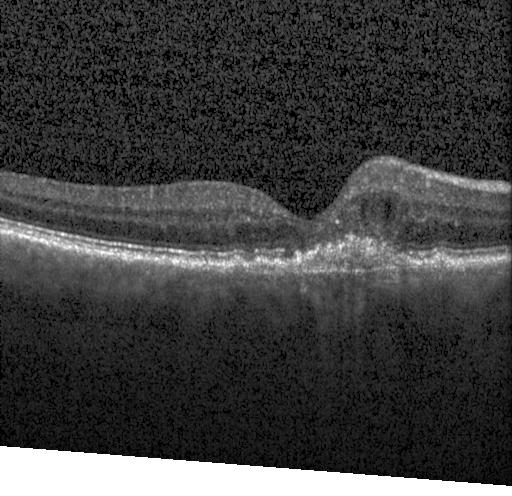
OCT B-scan; SD-OCT. Assessment: choroidal neovascularization.